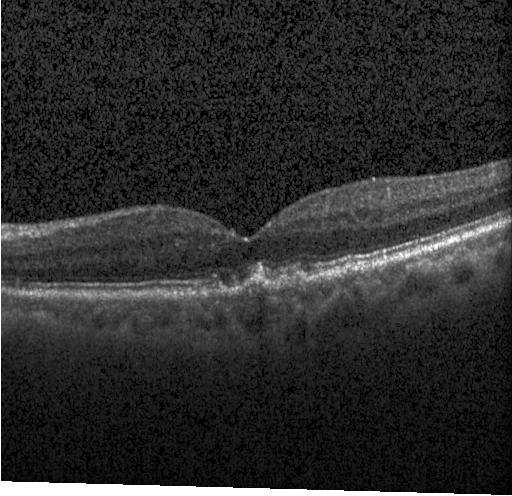
Spectral-domain optical coherence tomography · OCT B-scan. Multiple drusen.